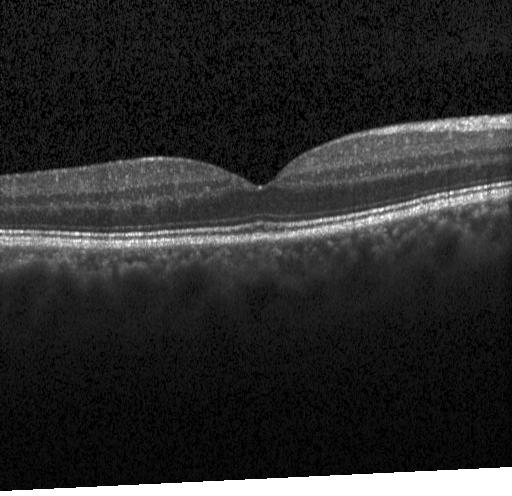
Impression: no choroidal neovascularization, no diabetic macular edema, and no drusen.